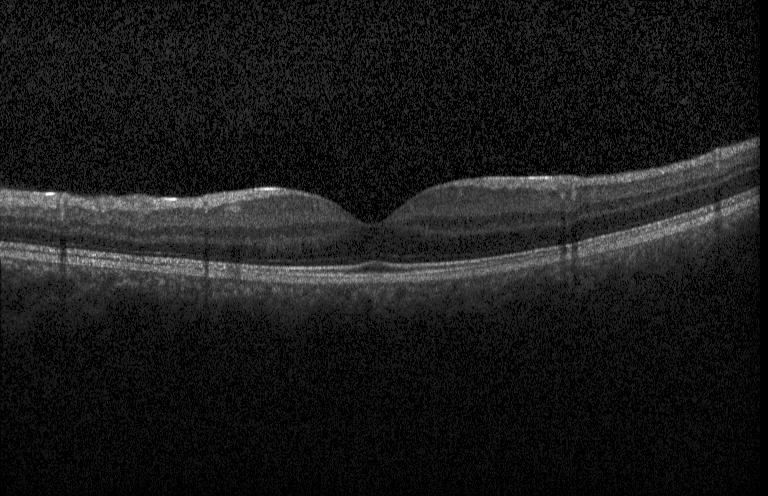
OCT B-scan, fovea-centered. Impression: no evidence of choroidal neovascularization, diabetic macular edema, or drusen.